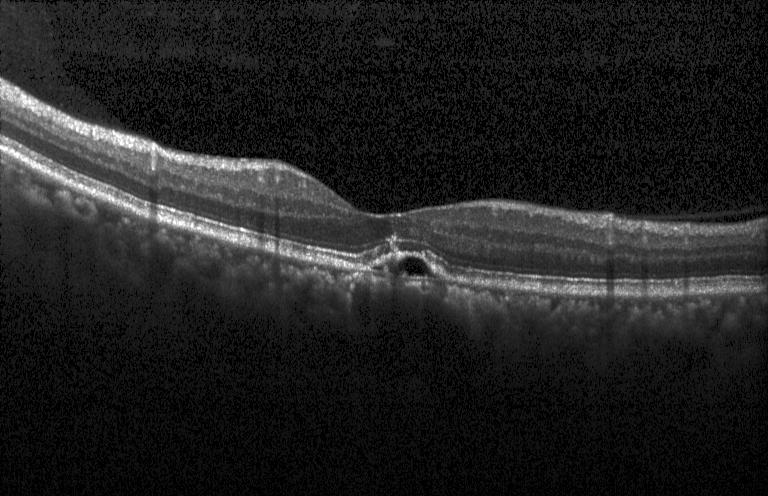 SD-OCT. Optical coherence tomography B-scan. Heidelberg Spectralis OCT system. Macular scan — Macular OCT: a choroidal neovascular membrane.